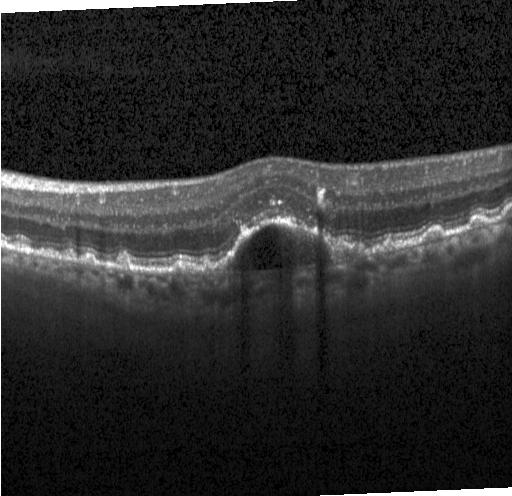

Diagnosis: a choroidal neovascular membrane.